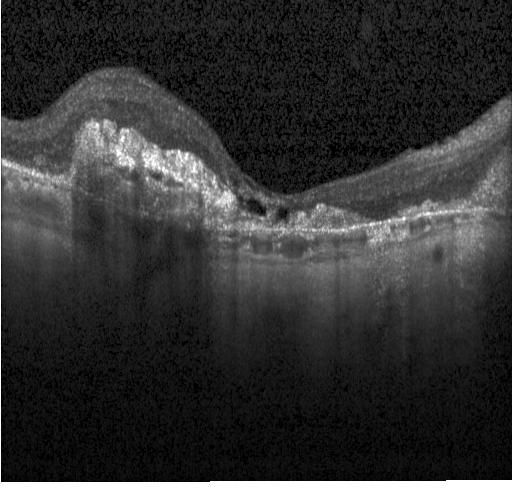
Dx: a choroidal neovascular membrane.